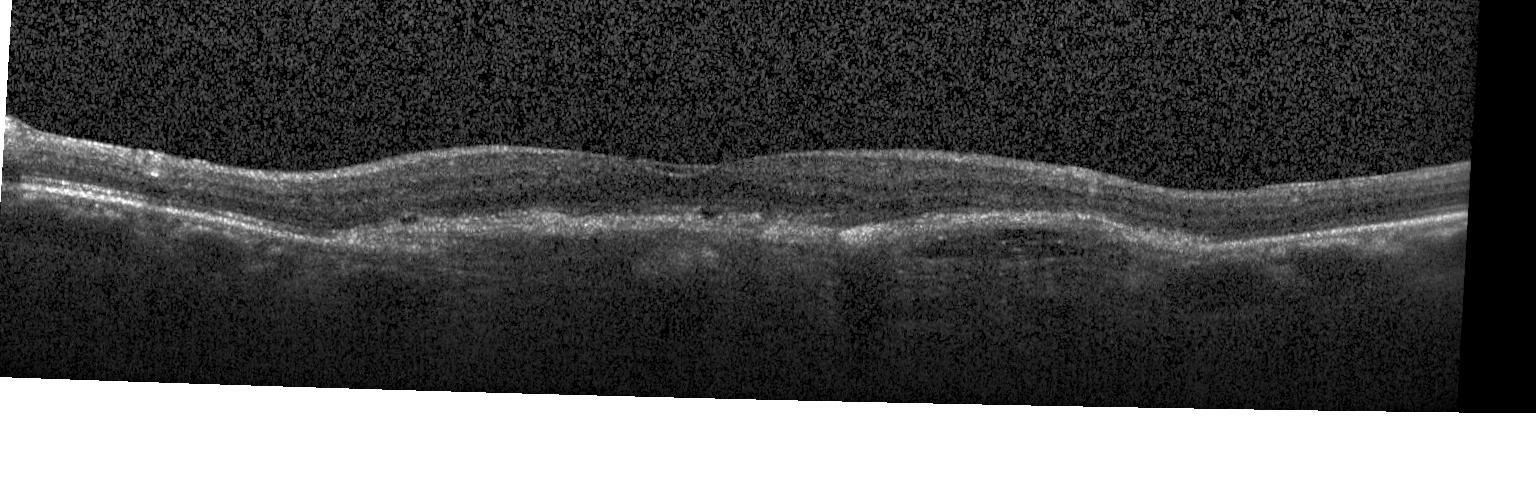
Assessment: a choroidal neovascular membrane.